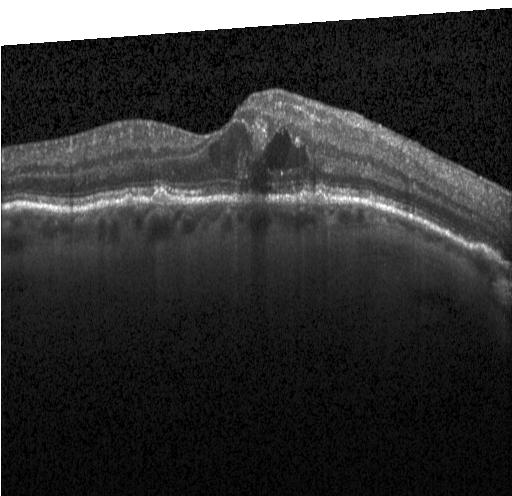
Optical coherence tomography B-scan. Assessment: choroidal neovascularization (CNV).